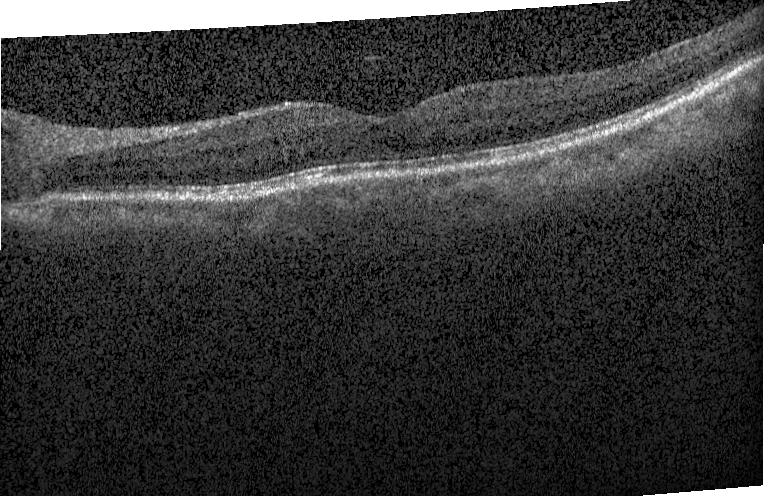

OCT line scan; spectral-domain OCT; centered on the fovea; Heidelberg Spectralis. The scan shows no CNV, DME, or drusen.